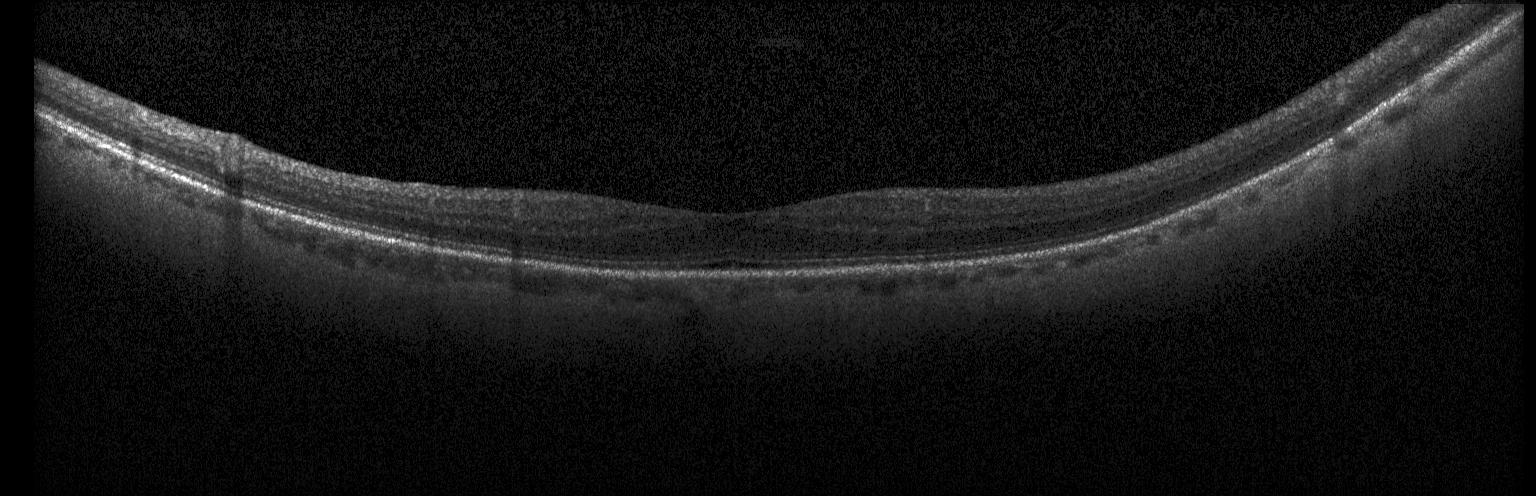

The scan shows no choroidal neovascularization, no diabetic macular edema, and no drusen.